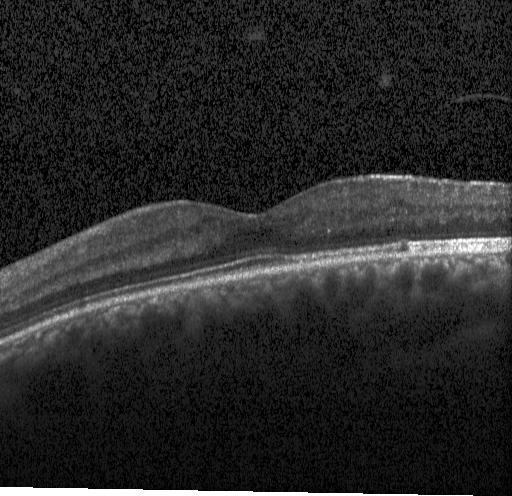
Fovea-centered · OCT B-scan. Diagnosis: no CNV, no DME, and no drusen.